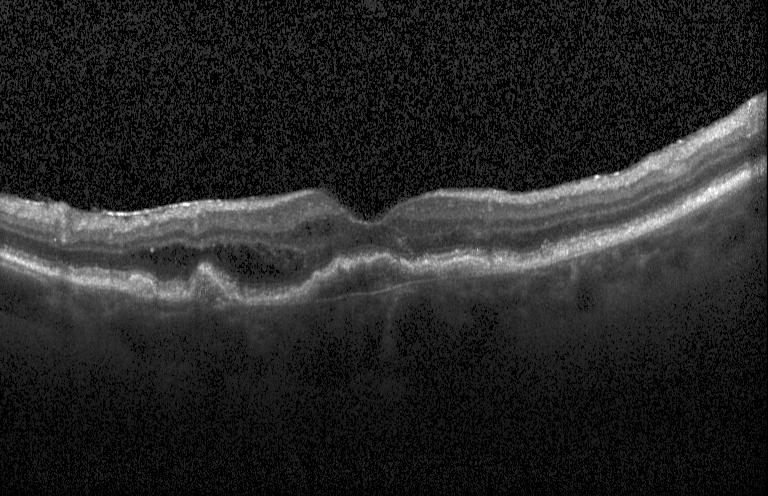

Optical coherence tomography scan, instrument: Heidelberg Spectralis, SD-OCT
Diagnosis: a choroidal neovascular membrane.